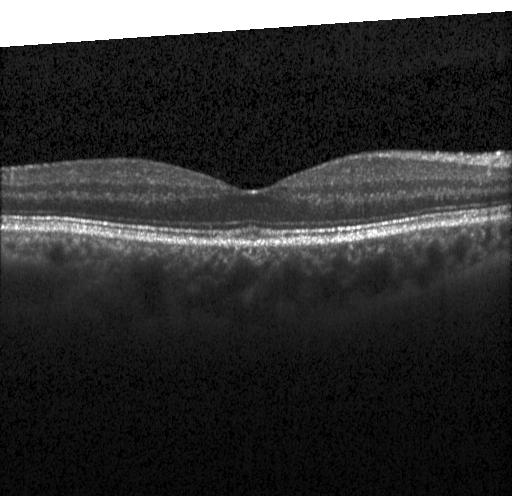

Optical coherence tomography B-scan
Finding: no CNV, DME, or drusen.